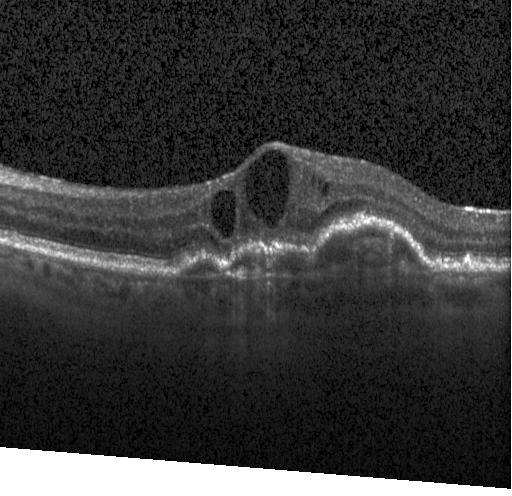

Diagnosis: a choroidal neovascular membrane.